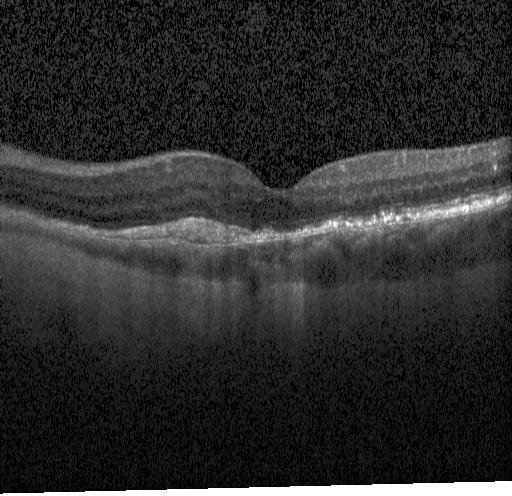

Acquired on a Heidelberg Spectralis, macular scan, OCT B-scan, spectral-domain OCT. The scan shows a choroidal neovascular membrane.